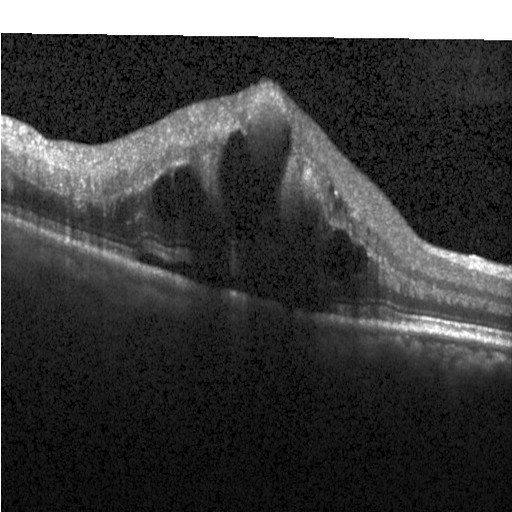 Diagnosis: diabetic macular edema.